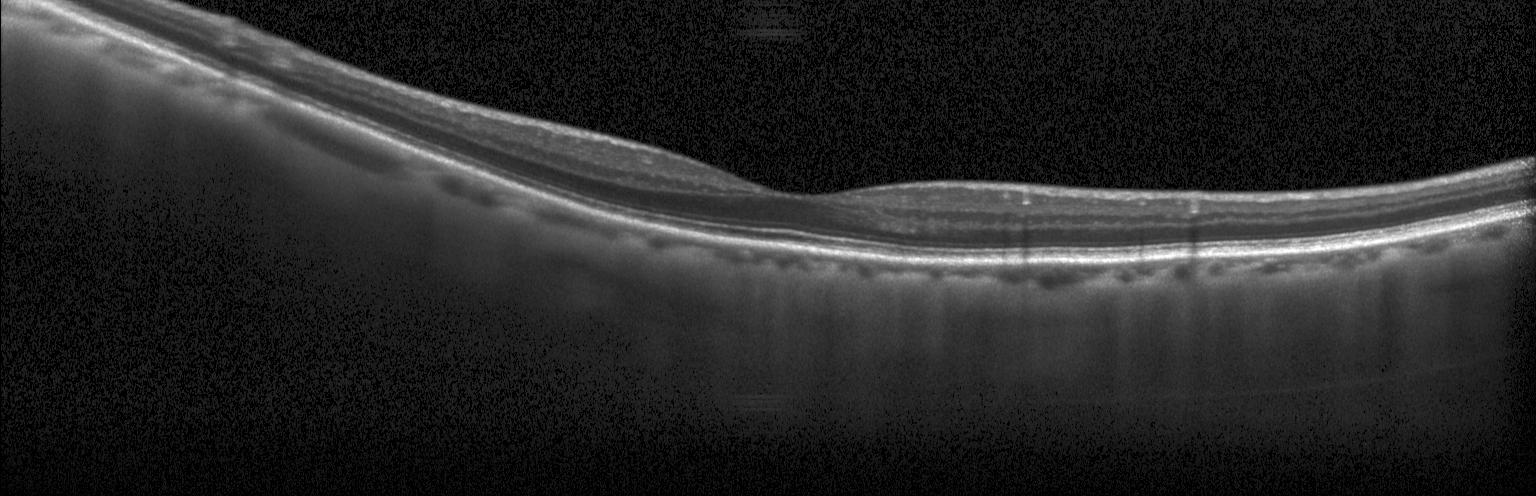 Macular OCT: no choroidal neovascularization, diabetic macular edema, or drusen.